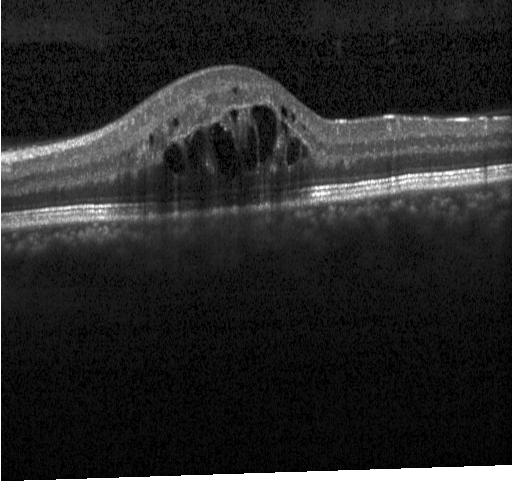

OCT B-scan showing diabetic macular edema.